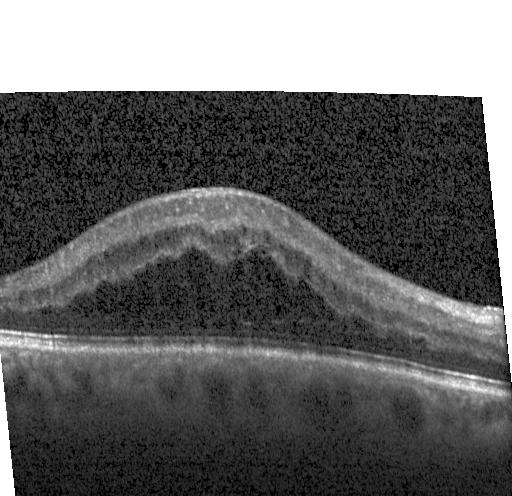 Macular OCT: DME.